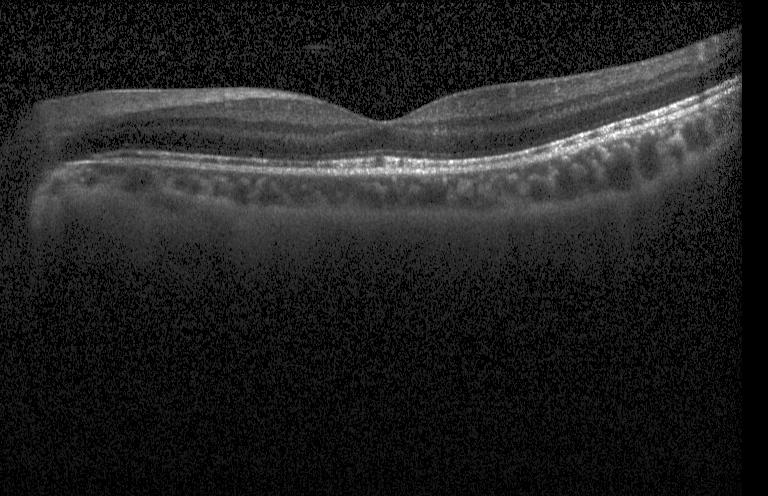

Finding: no choroidal neovascularization, diabetic macular edema, or drusen.